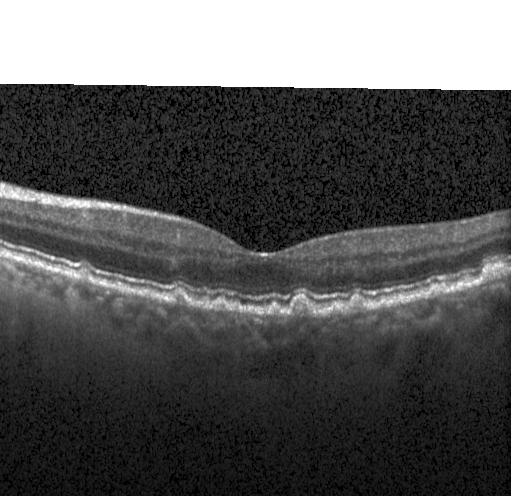

Spectral-domain OCT · OCT B-scan — The scan shows sub-RPE drusenoid deposits.